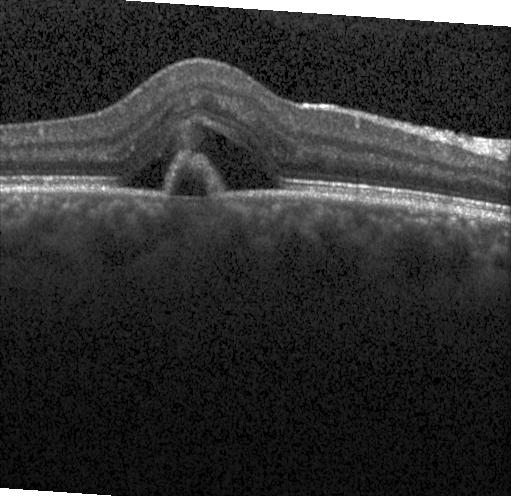
Finding: a choroidal neovascular membrane.